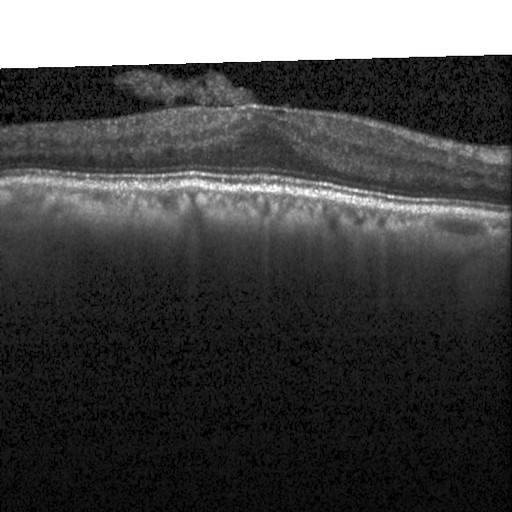 Centered on the fovea, retinal OCT B-scan, Heidelberg Spectralis, SD-OCT.
This B-scan demonstrates diabetic macular edema (DME).